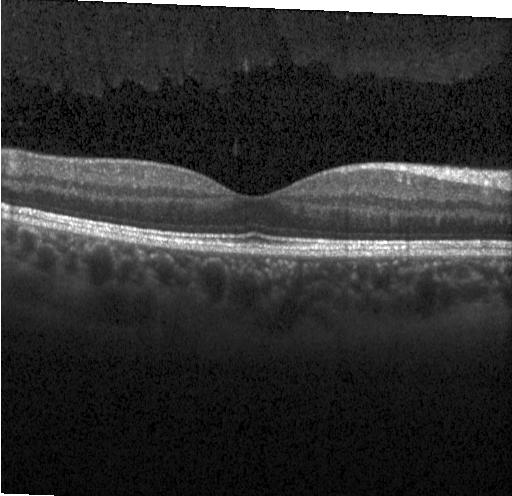
Spectral-domain optical coherence tomography; OCT line scan; fovea-centered.
Dx: no choroidal neovascularization, diabetic macular edema, or drusen.